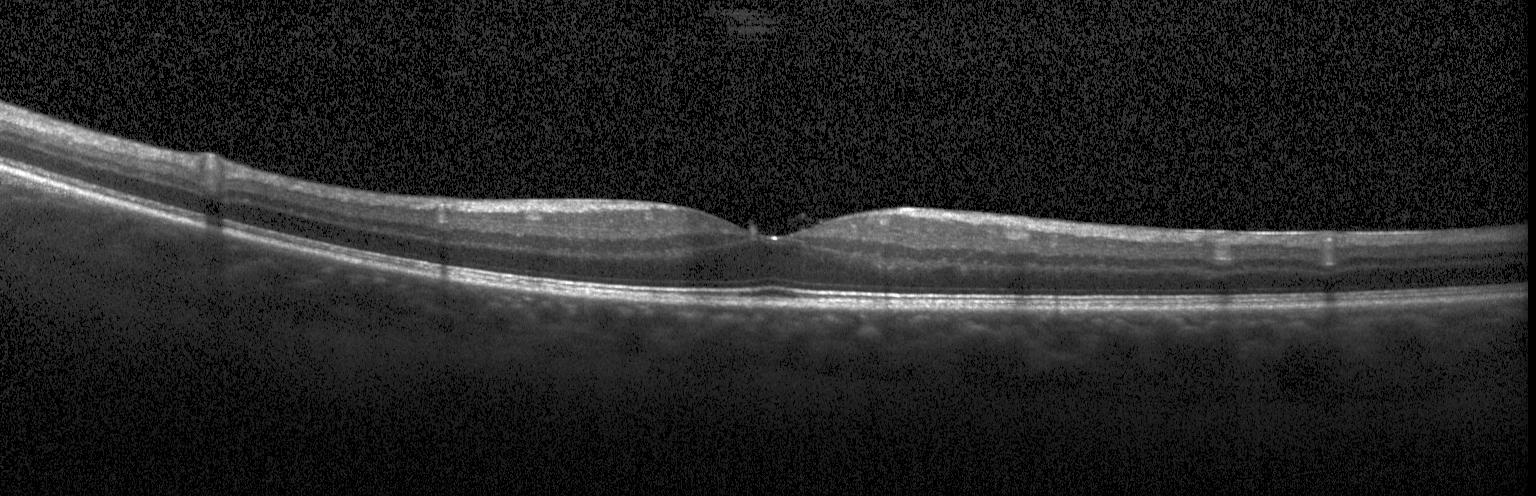
Retinal OCT cross-section. Dx: neither CNV, DME, nor drusen.